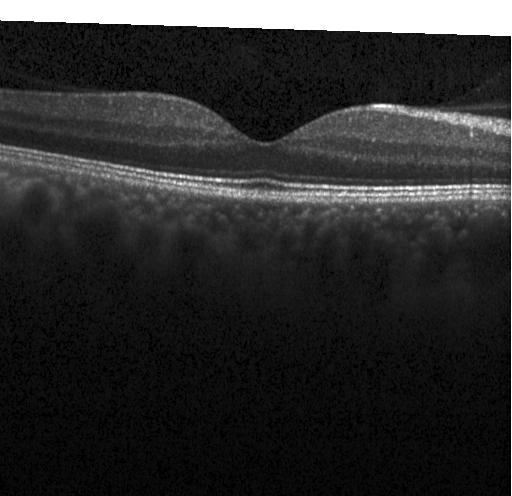

The scan shows neither choroidal neovascularization, diabetic macular edema, nor drusen.